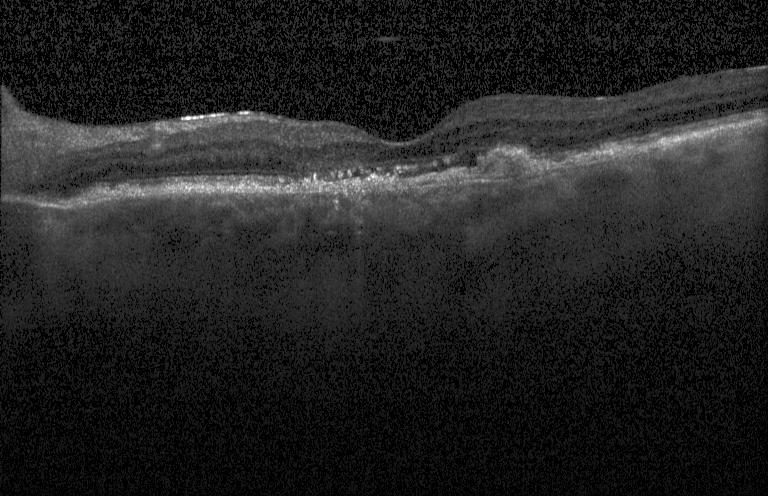
Heidelberg Spectralis OCT system · fovea-centered · retinal OCT B-scan.
OCT finding: a choroidal neovascular membrane.